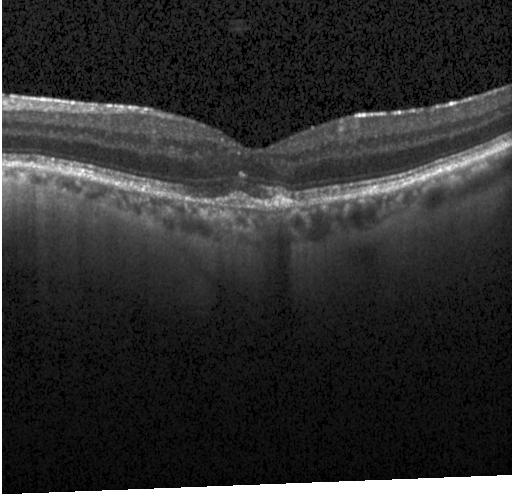 Macular OCT demonstrating a choroidal neovascular membrane.